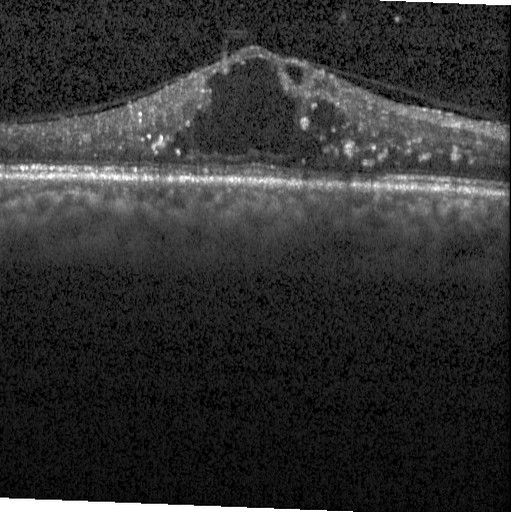

OCT B-scan showing diabetic macular edema (DME).